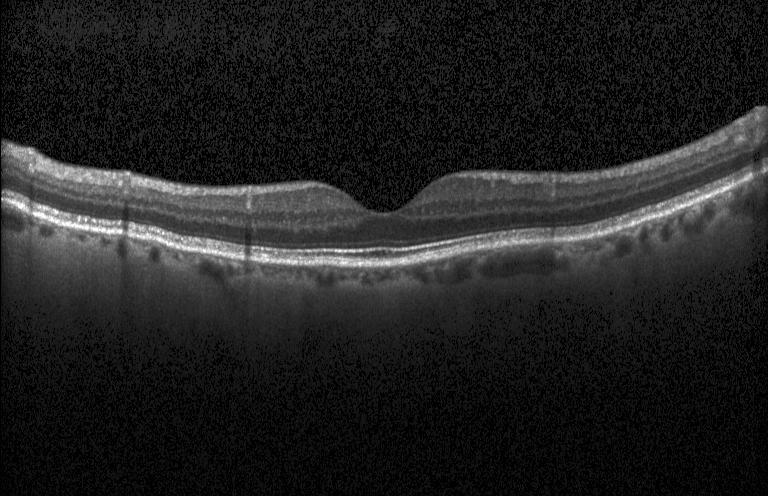
Instrument: Heidelberg Spectralis; OCT line scan
Impression: no CNV, no DME, and no drusen.